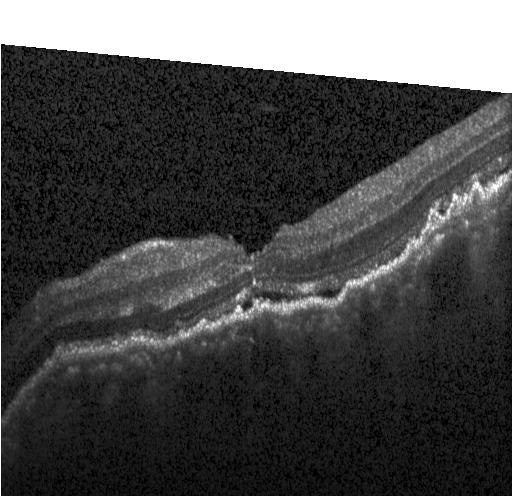
Dx: a choroidal neovascular membrane.